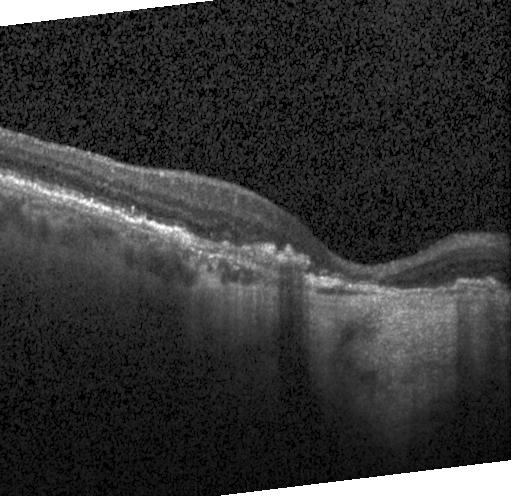

Retinal OCT cross-section
OCT finding: a choroidal neovascular membrane.